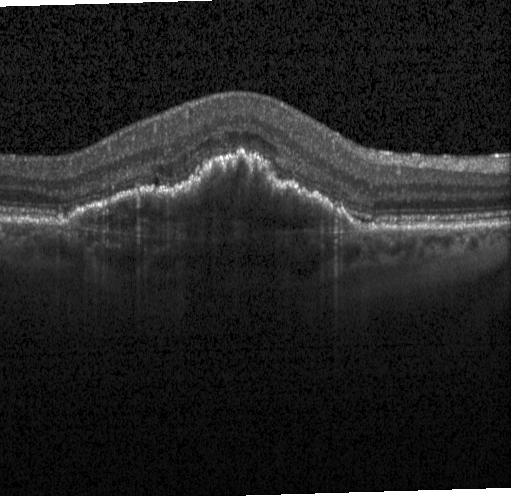
Spectral-domain OCT. Acquired on a Heidelberg Spectralis. OCT B-scan
Macular OCT: a choroidal neovascular membrane.